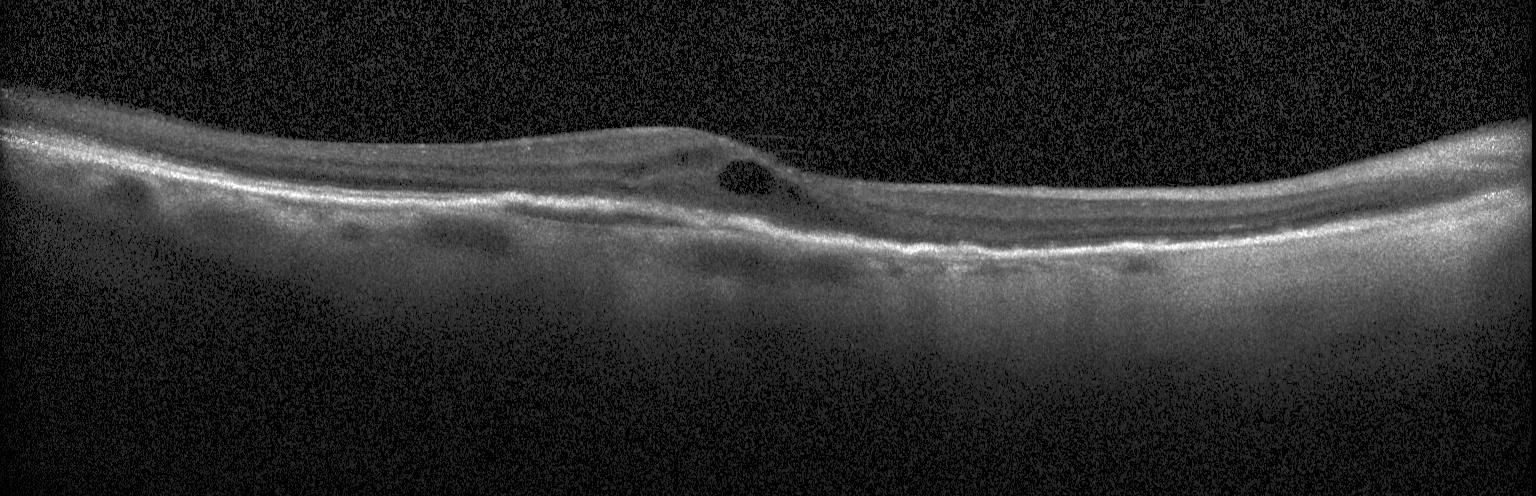 Spectral-domain OCT B-scan: a choroidal neovascular membrane.